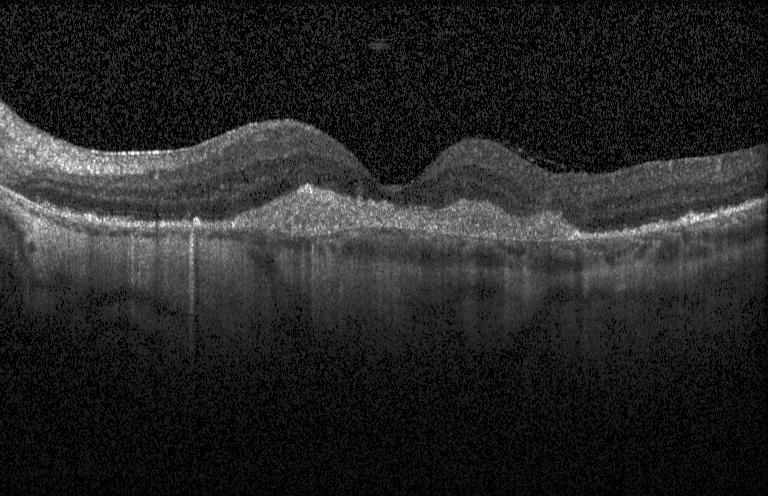 OCT line scan. Impression: choroidal neovascularization (CNV).